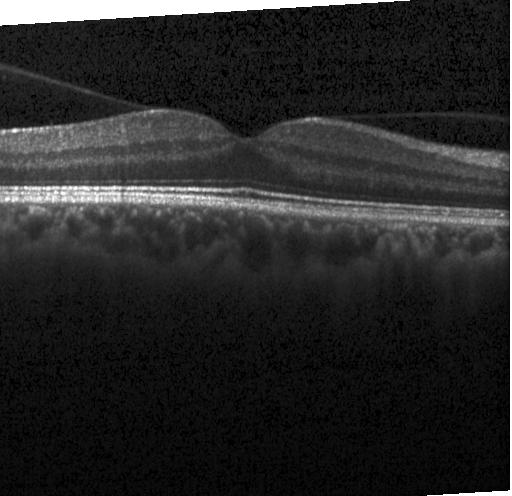

OCT B-scan showing no choroidal neovascularization, diabetic macular edema, or drusen.